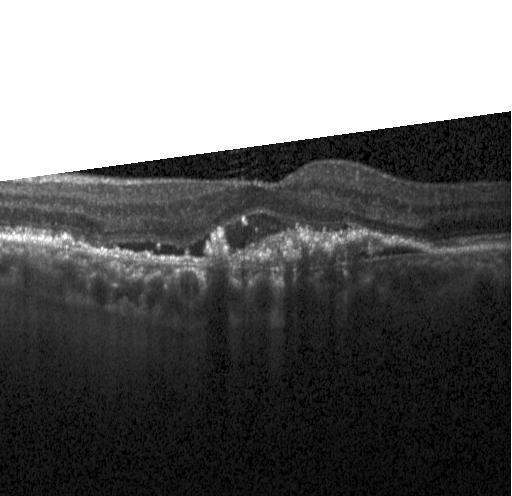

Finding: a choroidal neovascular membrane.